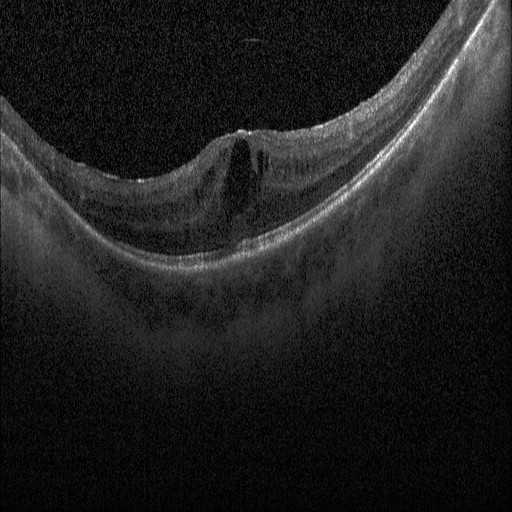
Optical coherence tomography scan · spectral-domain optical coherence tomography.
Diagnosis: diabetic macular edema (DME).